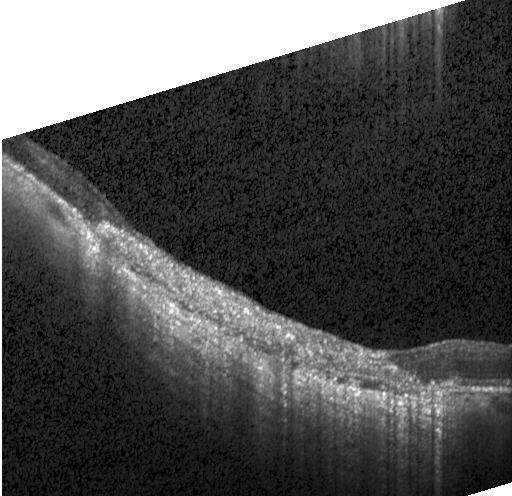 OCT B-scan.
Impression: a choroidal neovascular membrane.